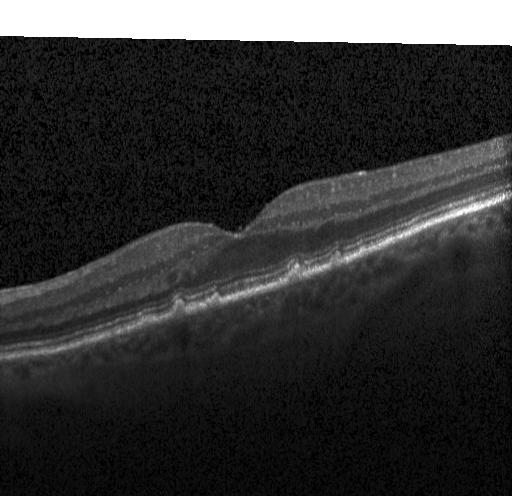

Fovea-centered; retinal OCT cross-section.
Assessment: drusen.